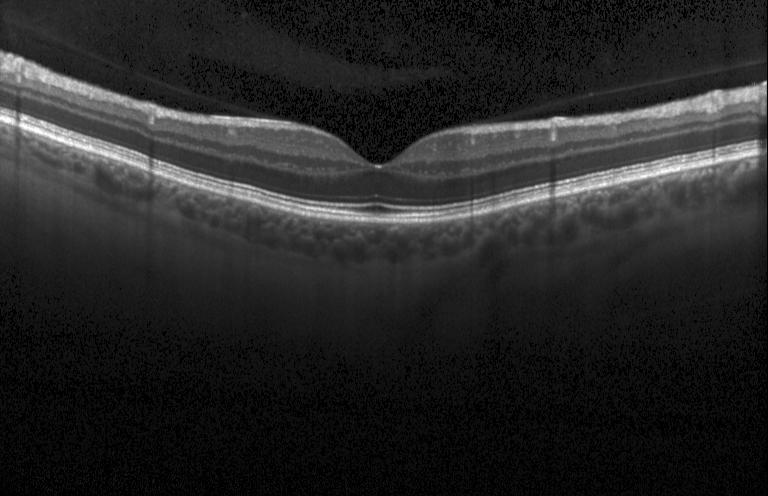 Retinal OCT cross-section showing no choroidal neovascularization, diabetic macular edema, or drusen.